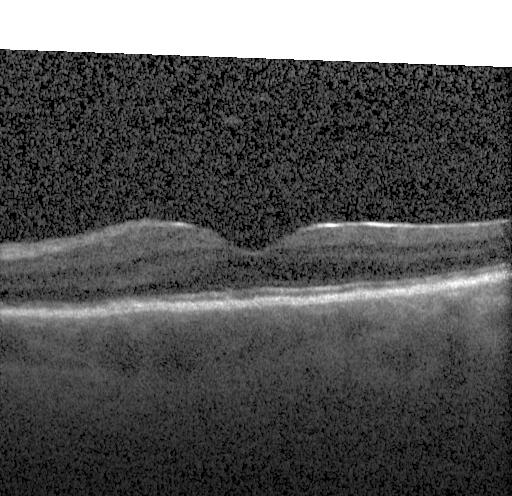 Impression: no choroidal neovascularization, no diabetic macular edema, and no drusen.